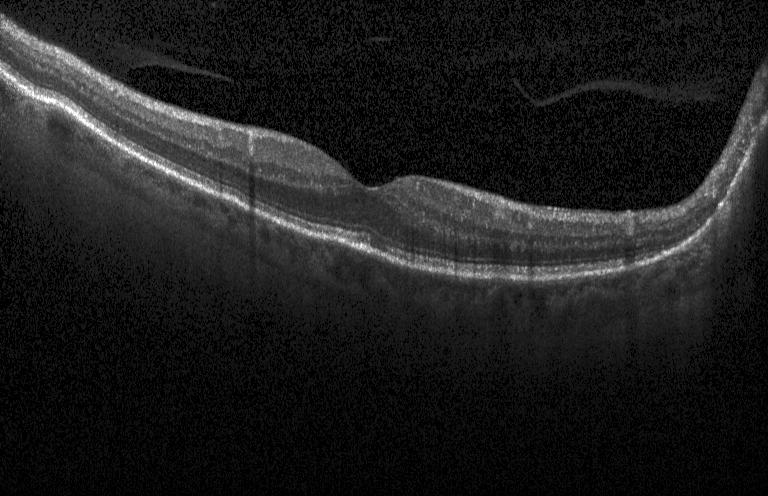
Optical coherence tomography B-scan · Heidelberg Spectralis.
Assessment: no choroidal neovascularization, no diabetic macular edema, and no drusen.